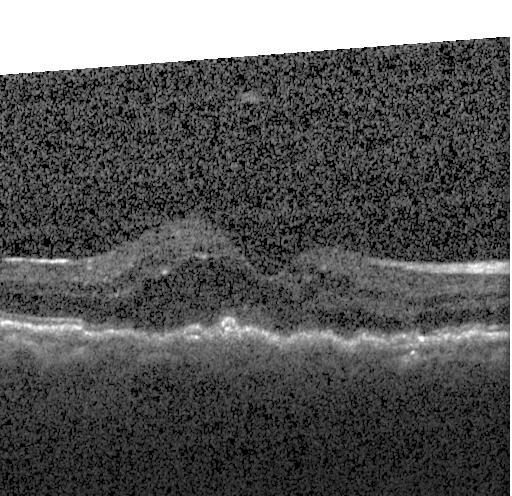
Retinal OCT cross-section showing choroidal neovascularization (CNV).